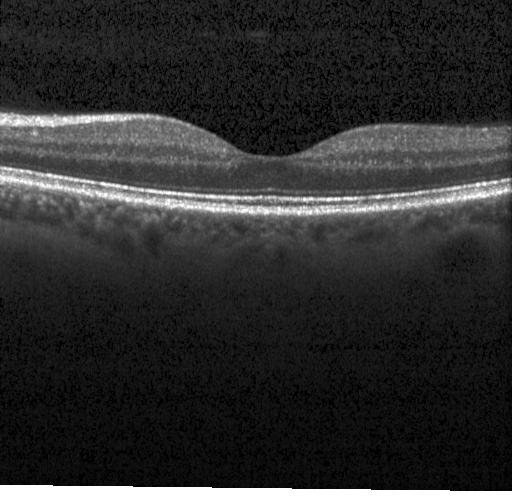
Diagnosis: neither CNV, DME, nor drusen.